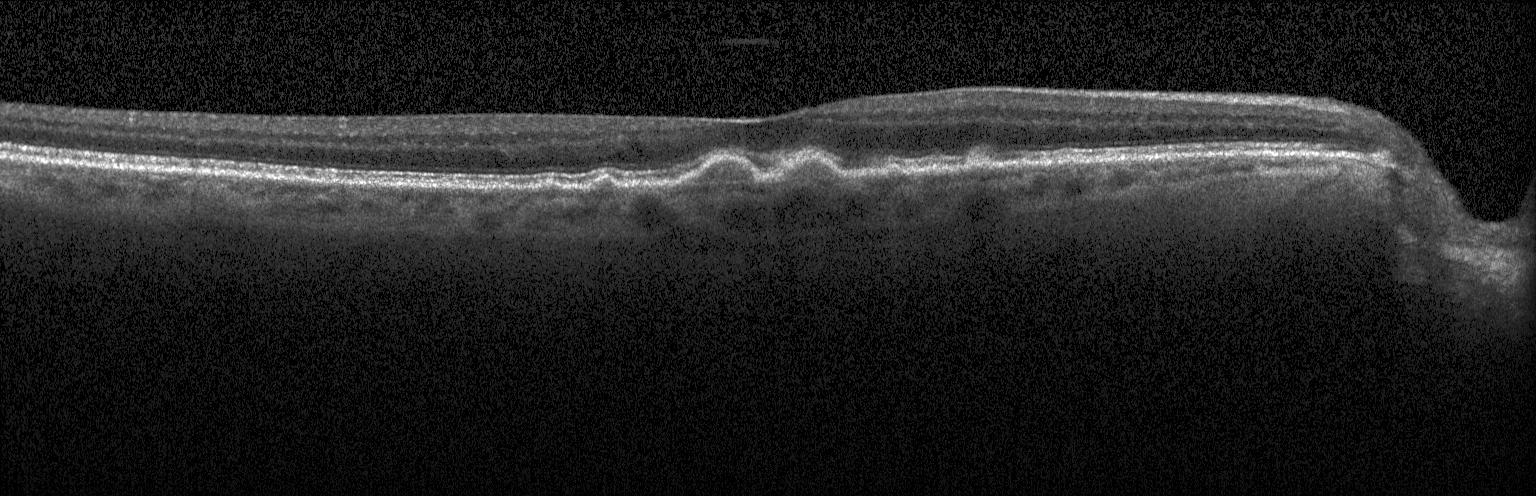

Diagnosis: multiple drusen.